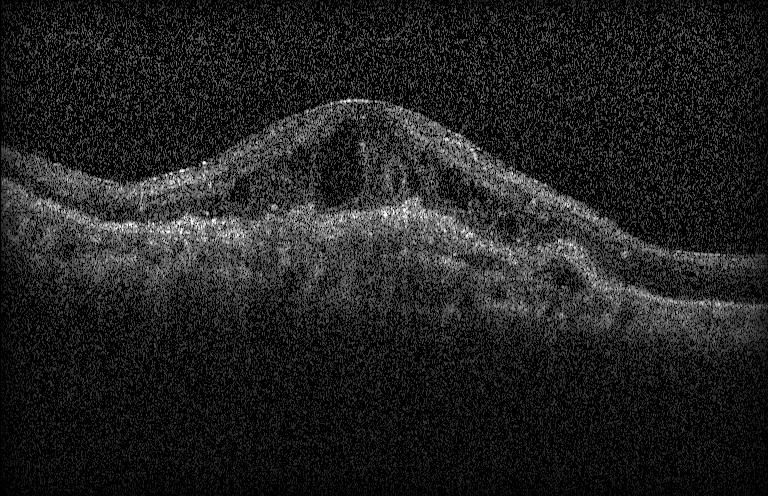

OCT scan showing a choroidal neovascular membrane.